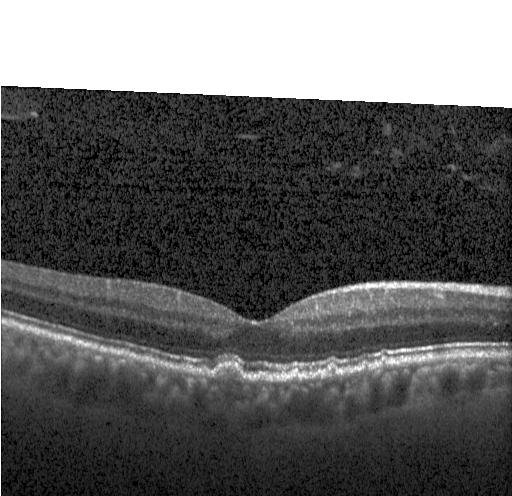
Retinal OCT B-scan. Spectral-domain optical coherence tomography. Finding: drusen.